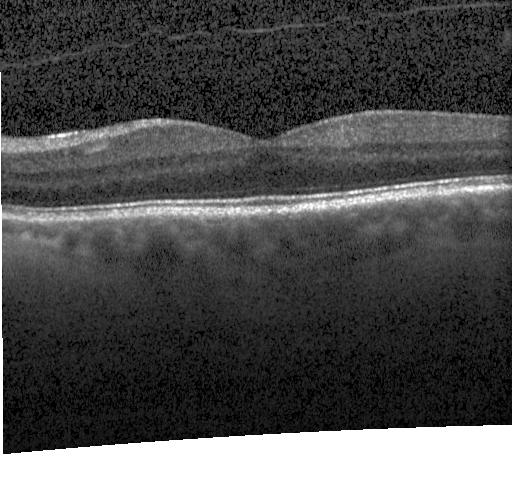 Finding: no CNV, DME, or drusen.